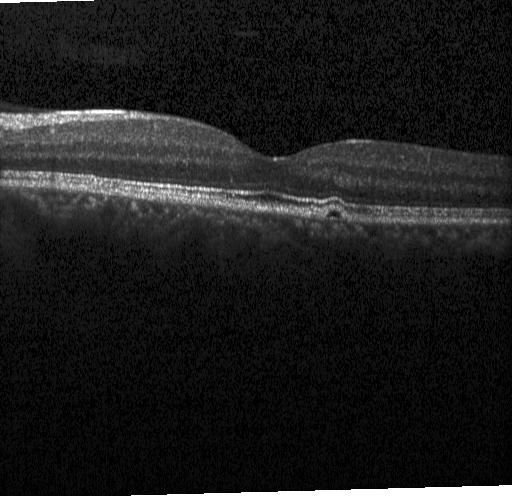

Dx: sub-RPE drusenoid deposits.